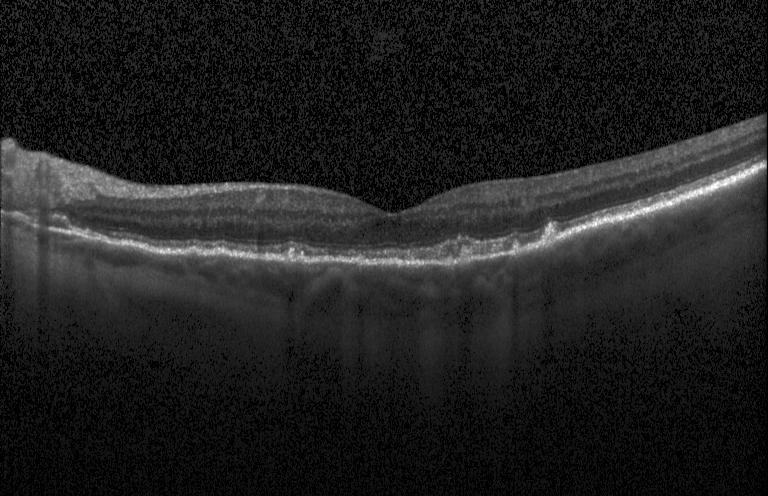 Through the macula; spectral-domain optical coherence tomography; Heidelberg Spectralis OCT system; retinal OCT cross-section — Impression: drusen.